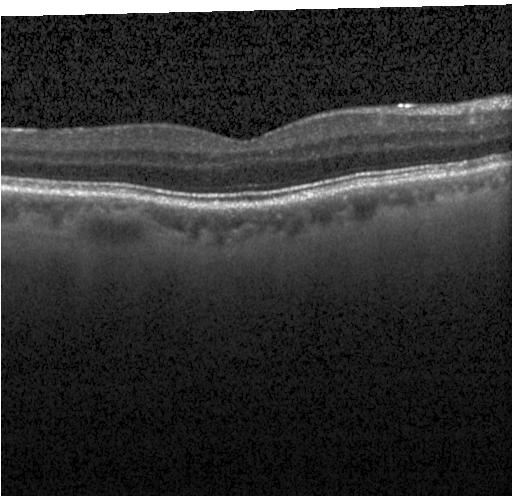
This B-scan demonstrates no choroidal neovascularization, diabetic macular edema, or drusen.